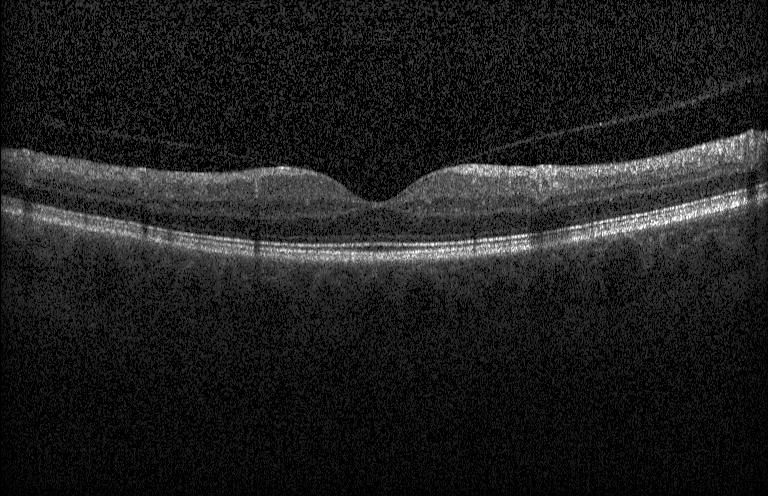
Through the macula · instrument: Heidelberg Spectralis · OCT B-scan · spectral-domain OCT
Finding: no CNV, no DME, and no drusen.